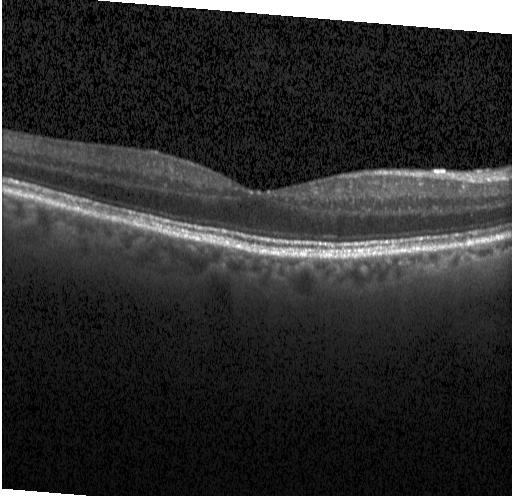 Spectral-domain optical coherence tomography, optical coherence tomography B-scan, instrument: Heidelberg Spectralis, through the macula
Macular OCT: no CNV, no DME, and no drusen.